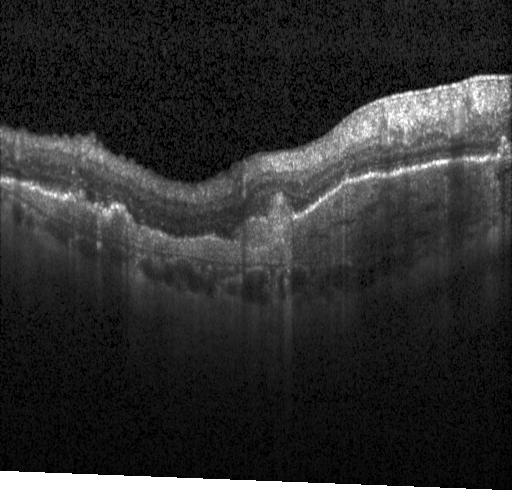
SD-OCT, acquired on a Heidelberg Spectralis, horizontal scan through the fovea, OCT line scan.
Choroidal neovascularization (CNV).